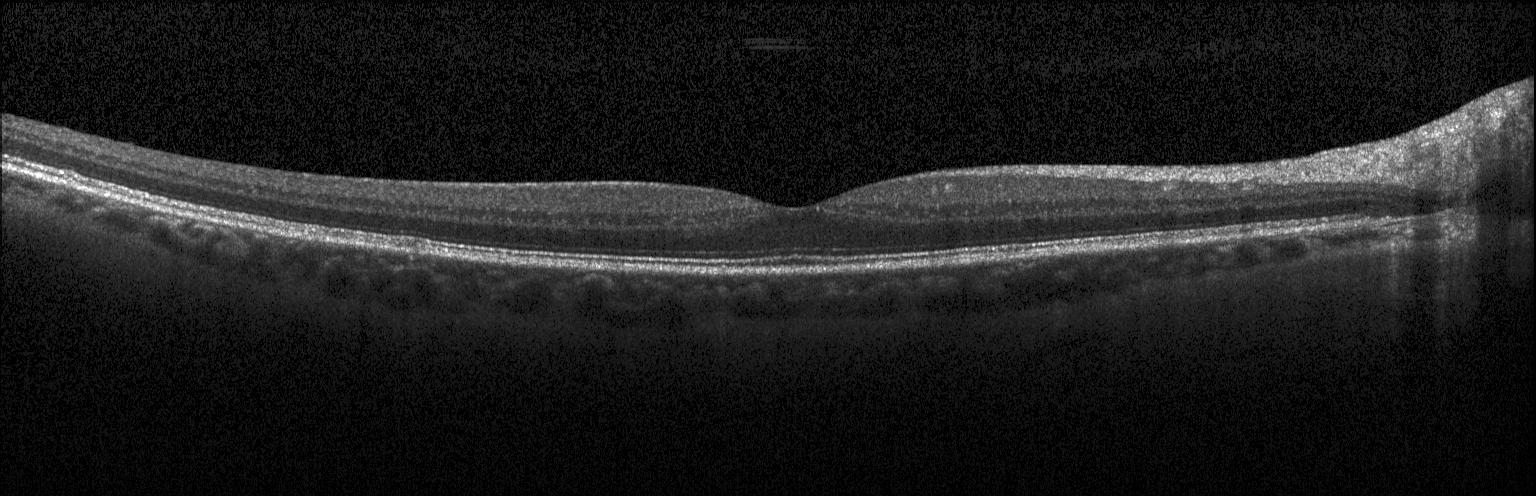
Diagnosis: neither CNV, DME, nor drusen.